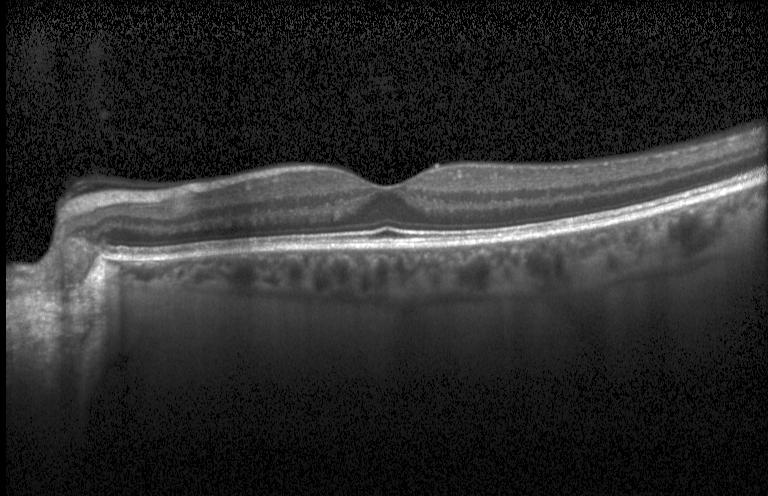
Retinal OCT B-scan. SD-OCT.
Impression: neither choroidal neovascularization, diabetic macular edema, nor drusen.